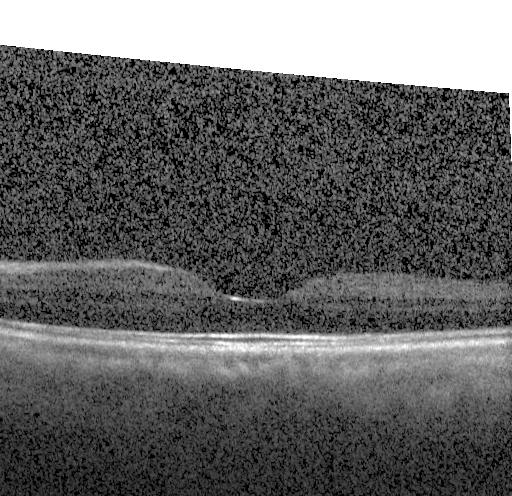
OCT B-scan; acquired on a Heidelberg Spectralis. This B-scan demonstrates no CNV, no DME, and no drusen.